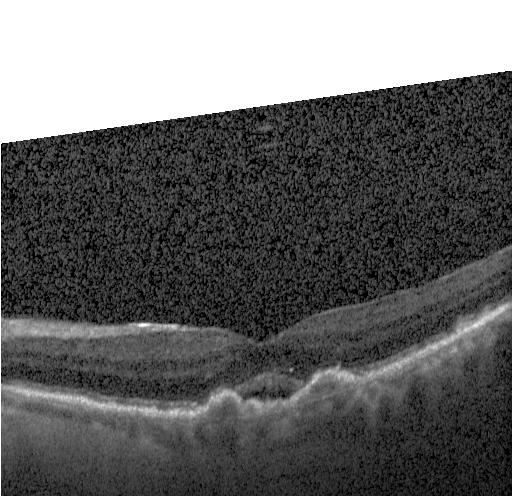

Centered on the fovea. Acquired on a Heidelberg Spectralis. OCT line scan. Finding: a choroidal neovascular membrane.